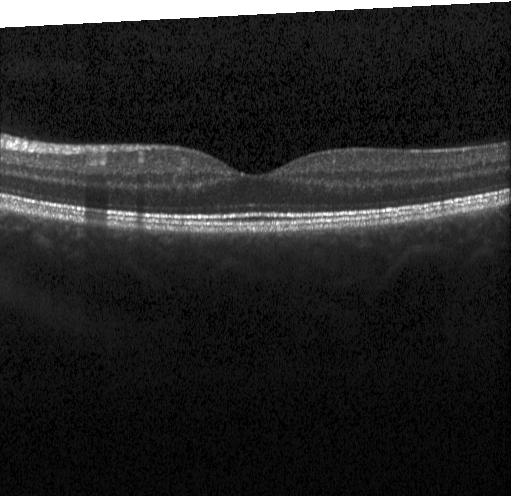

Retinal OCT cross-section — Impression: no evidence of choroidal neovascularization, diabetic macular edema, or drusen.